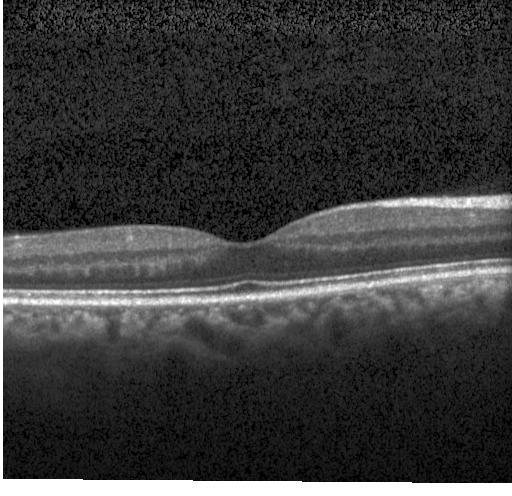

Assessment: no CNV, no DME, and no drusen.